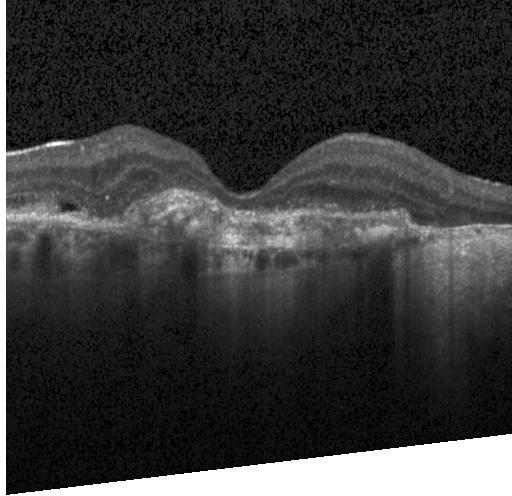
Spectral-domain OCT B-scan: a choroidal neovascular membrane.